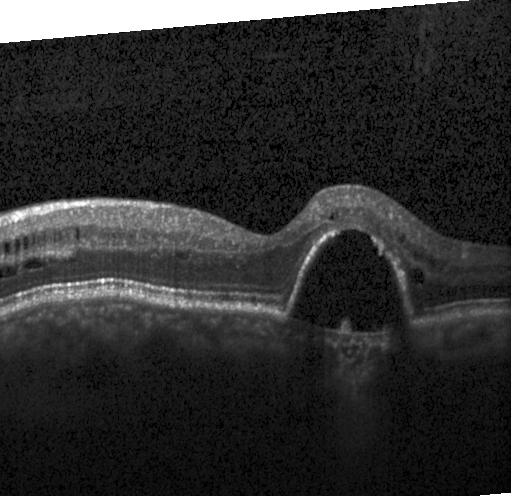

Spectral-domain optical coherence tomography; Heidelberg Spectralis; horizontal scan through the fovea; retinal OCT B-scan
Impression: a choroidal neovascular membrane.